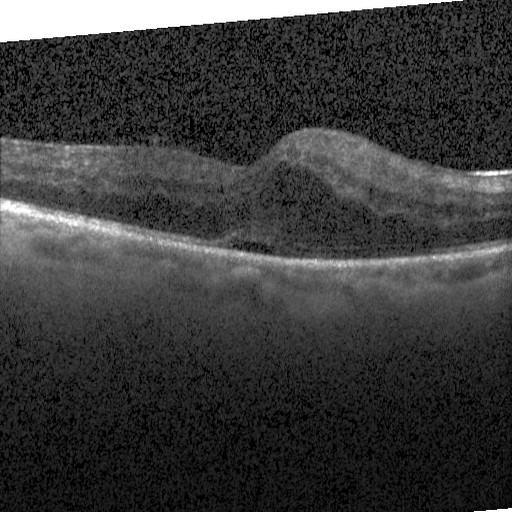

This B-scan demonstrates diabetic macular edema.